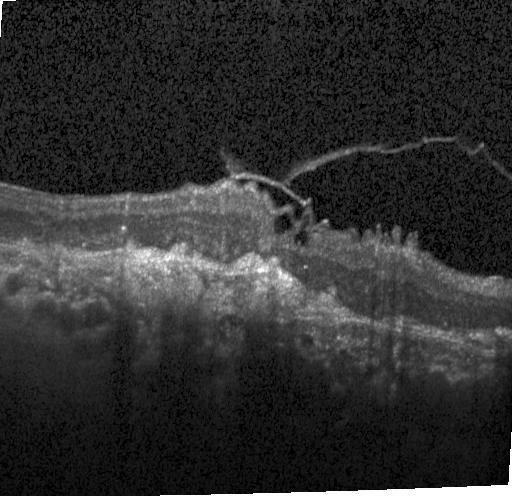

Heidelberg Spectralis · SD-OCT · optical coherence tomography B-scan
Diagnosis: a choroidal neovascular membrane.